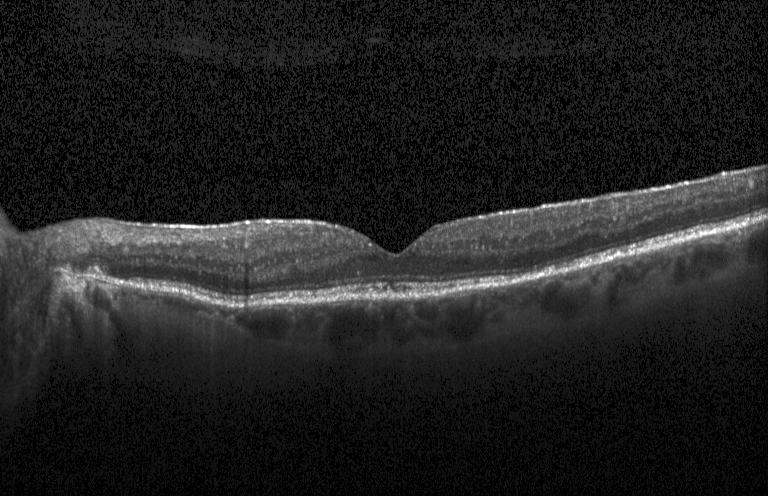 Dx: no CNV, no DME, and no drusen.